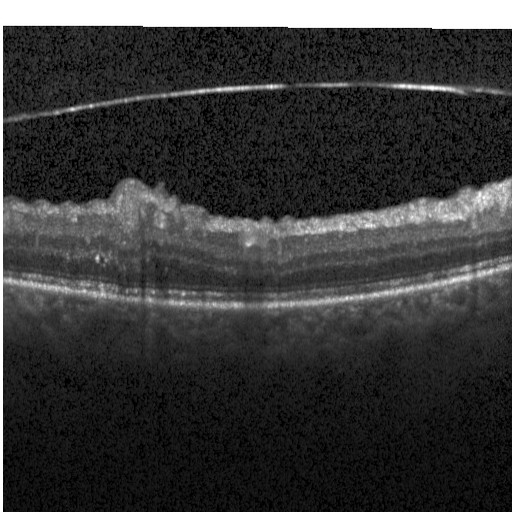 Optical coherence tomography B-scan. Impression: diabetic macular edema (DME).